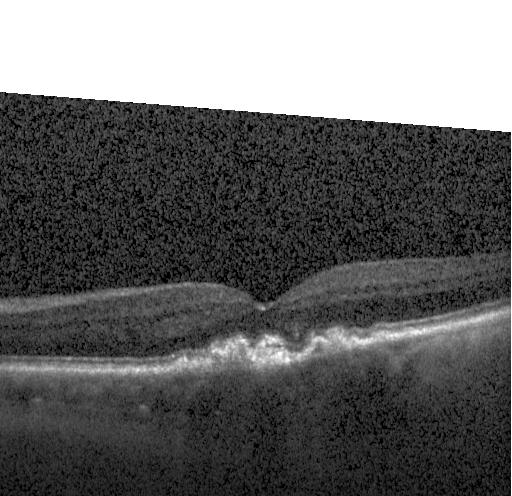
Finding: a choroidal neovascular membrane.